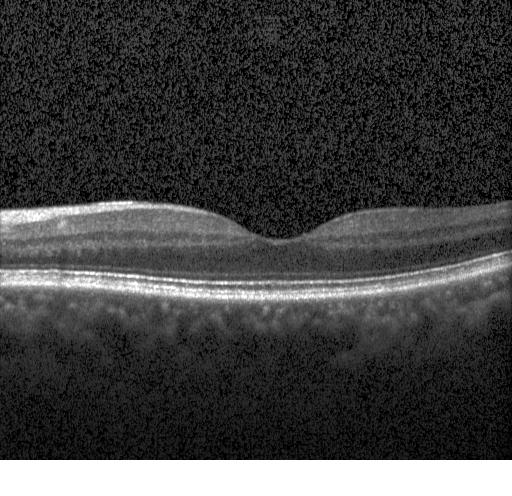
Instrument: Heidelberg Spectralis · OCT line scan. Assessment: neither CNV, DME, nor drusen.